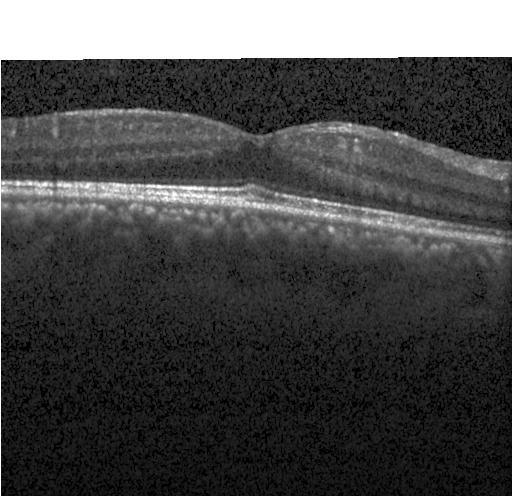 Dx: no CNV, no DME, and no drusen.